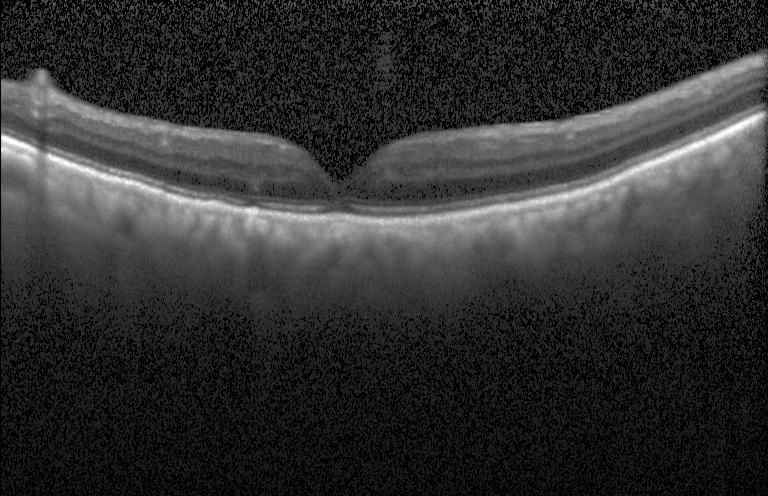 OCT B-scan. Assessment: no evidence of choroidal neovascularization, diabetic macular edema, or drusen.